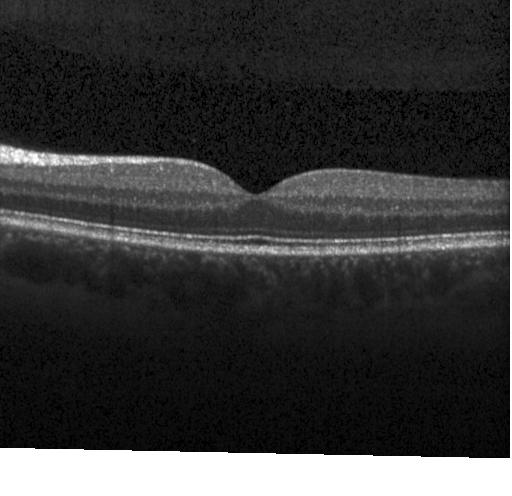
OCT B-scan showing no CNV, no DME, and no drusen.